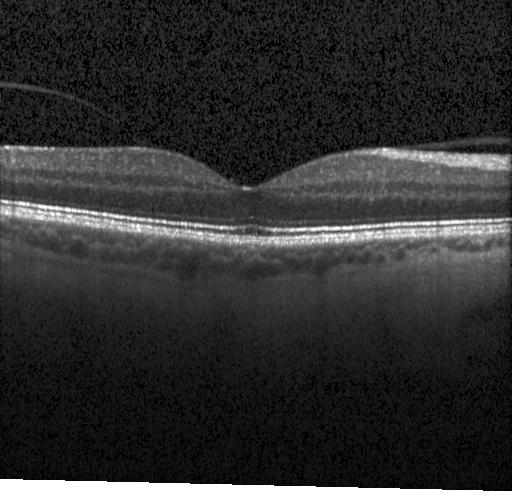 Centered on the fovea. Retinal OCT B-scan. Heidelberg Spectralis. SD-OCT. The scan shows neither choroidal neovascularization, diabetic macular edema, nor drusen.